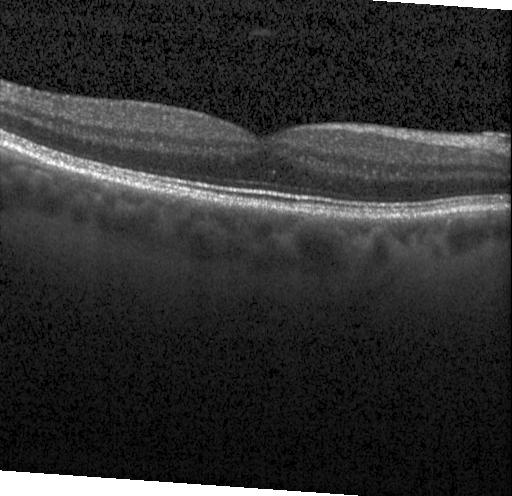 Impression: neither CNV, DME, nor drusen.